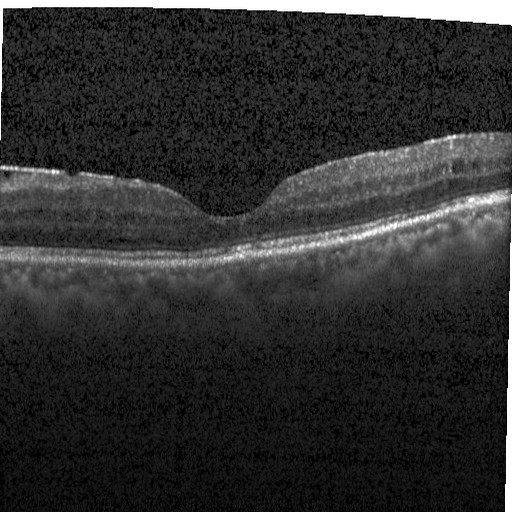
Optical coherence tomography B-scan. Impression: diabetic macular edema (DME).